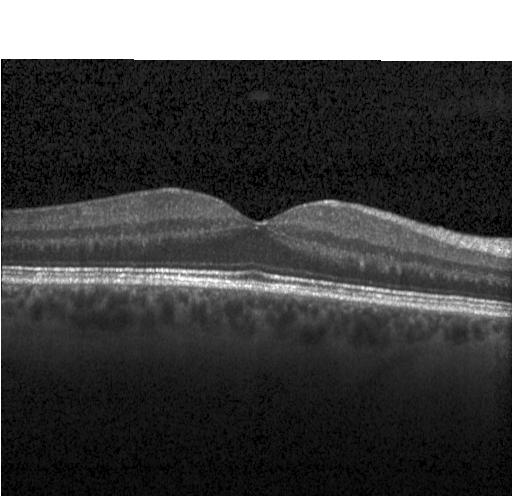
Spectral-domain optical coherence tomography · instrument: Heidelberg Spectralis · OCT B-scan · fovea-centered.
Diagnosis: no evidence of CNV, DME, or drusen.